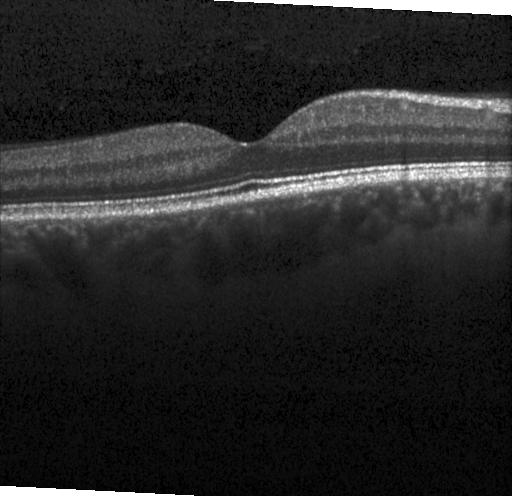

Centered on the fovea. Spectral-domain optical coherence tomography. OCT line scan. Instrument: Heidelberg Spectralis
The scan shows no choroidal neovascularization, no diabetic macular edema, and no drusen.